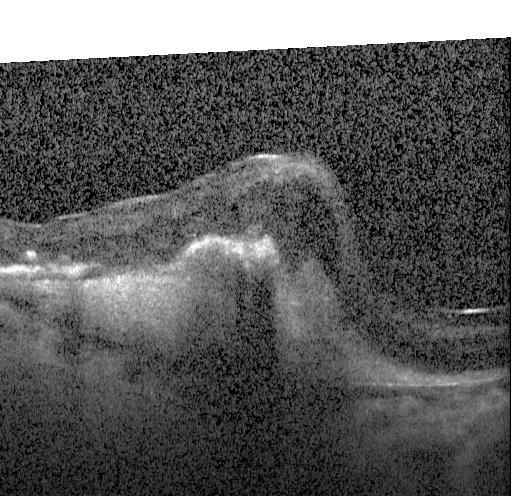 Retinal OCT cross-section; spectral-domain optical coherence tomography
Macular OCT: choroidal neovascularization (CNV).